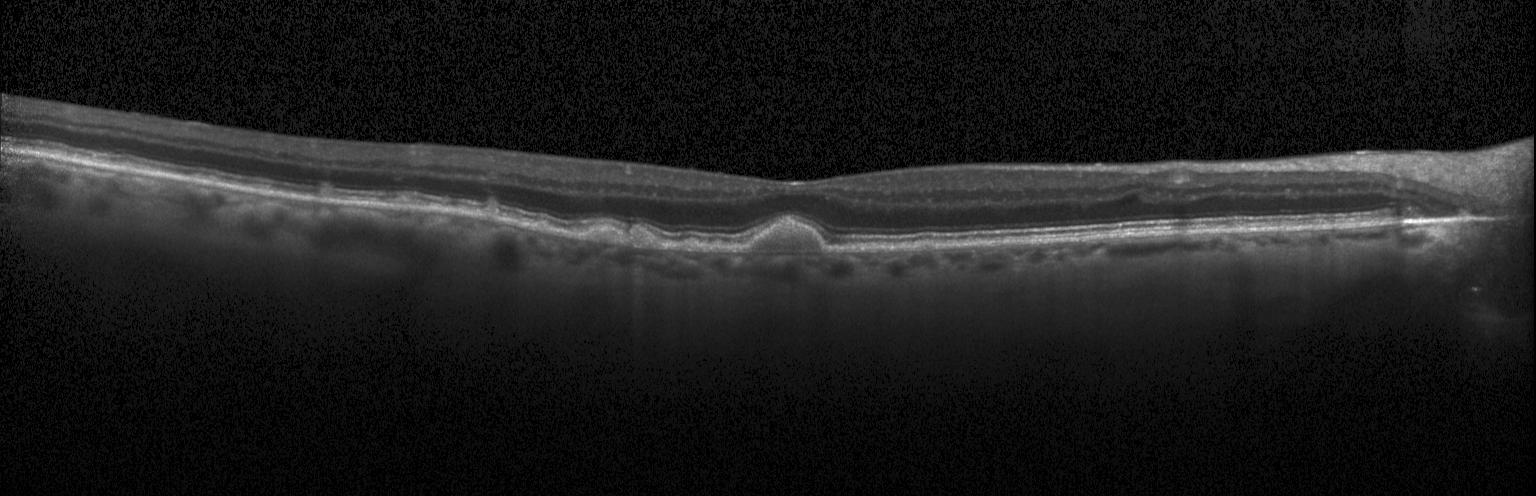
Macular OCT: sub-RPE drusenoid deposits.